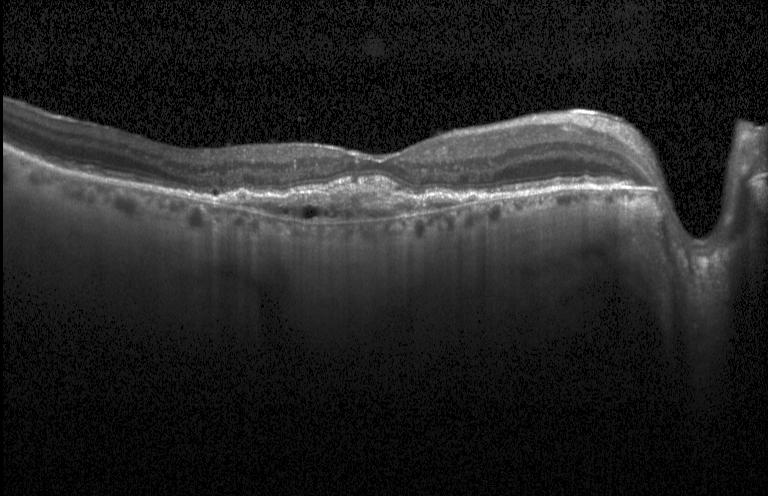

Dx: a choroidal neovascular membrane.